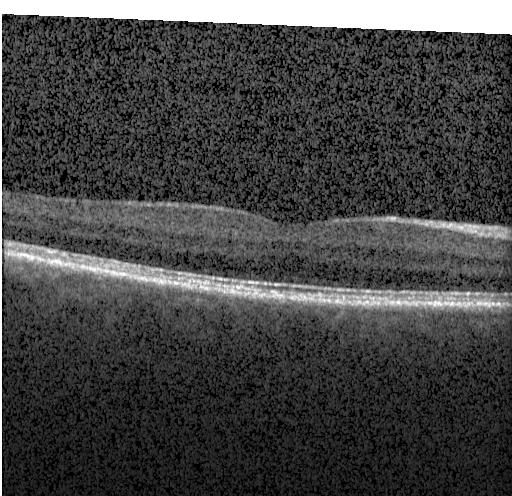
Retinal OCT B-scan.
Impression: no choroidal neovascularization, no diabetic macular edema, and no drusen.